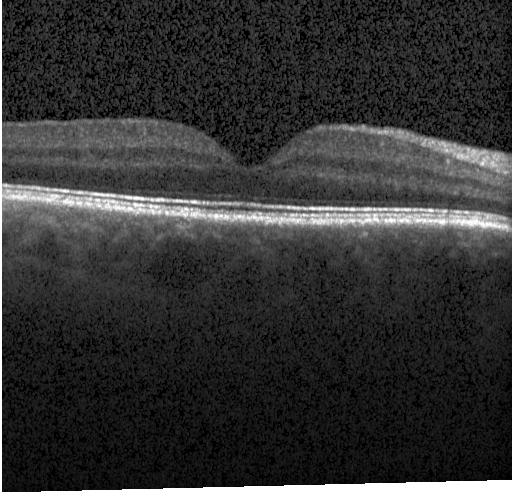

Horizontal scan through the fovea; retinal OCT B-scan; Heidelberg Spectralis.
This B-scan demonstrates no choroidal neovascularization, no diabetic macular edema, and no drusen.